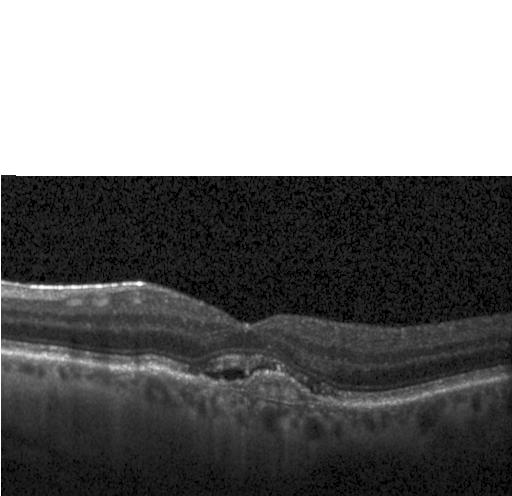 Retinal OCT B-scan — Impression: a choroidal neovascular membrane.